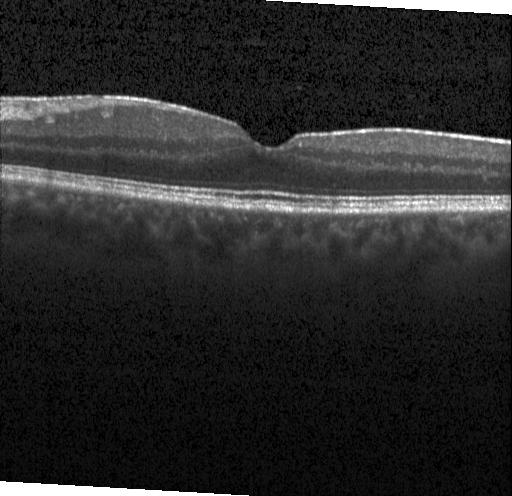 Diagnosis: no CNV, DME, or drusen.